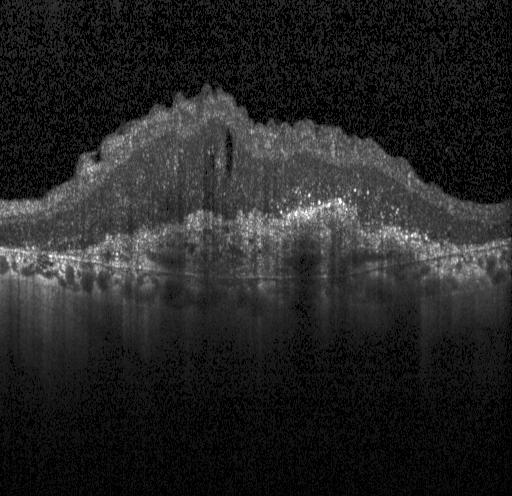
Heidelberg Spectralis · macular scan · OCT B-scan
Dx: choroidal neovascularization (CNV).